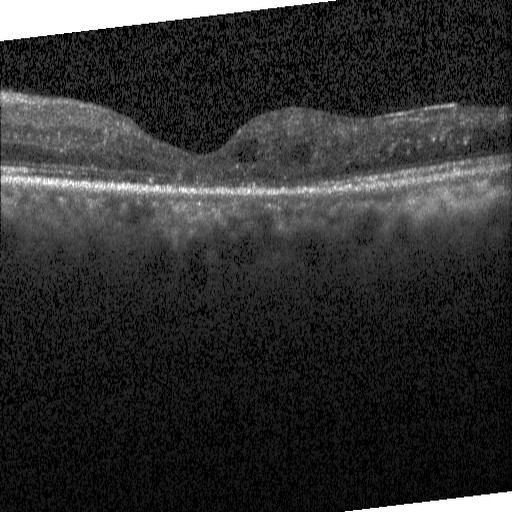

Instrument: Heidelberg Spectralis. Optical coherence tomography B-scan. Horizontal scan through the fovea
Impression: DME.